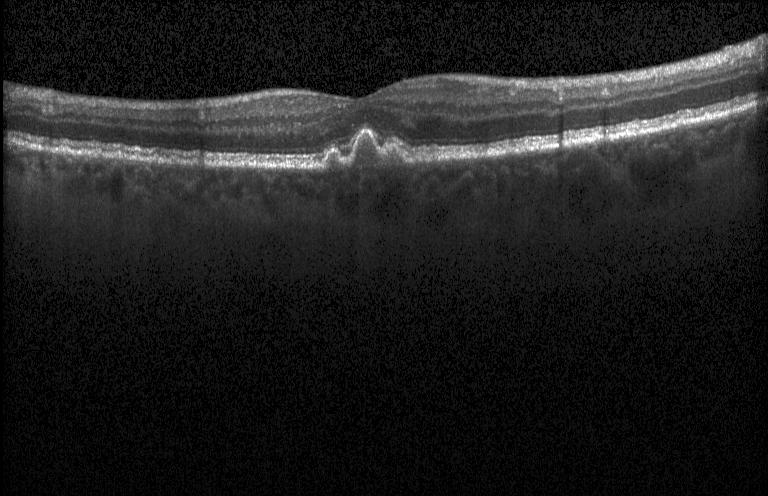 Diagnosis: sub-RPE drusenoid deposits.